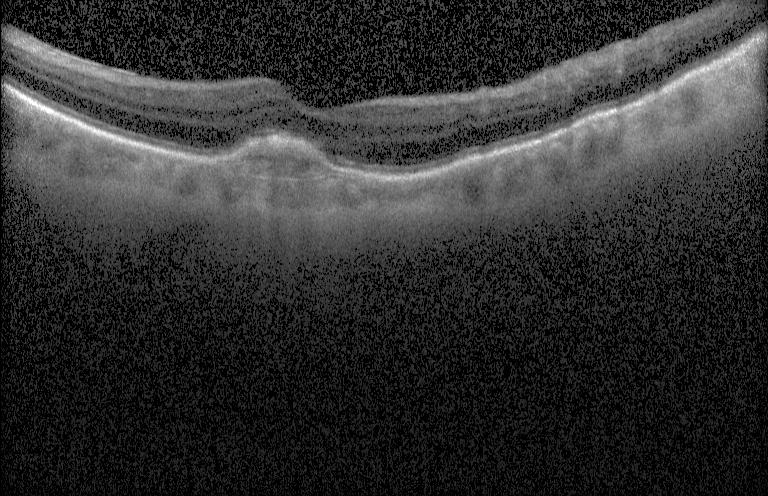
Optical coherence tomography scan — Assessment: choroidal neovascularization (CNV).